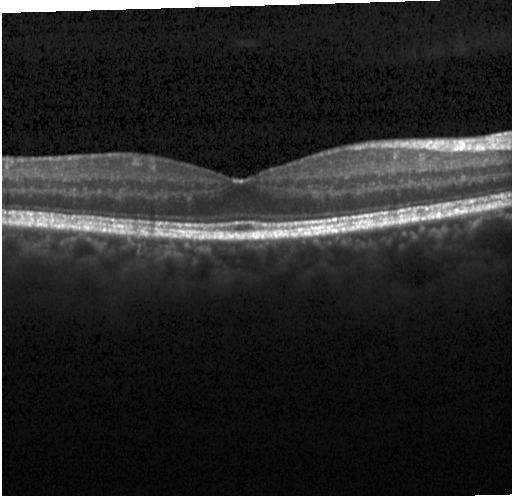 The scan shows neither CNV, DME, nor drusen.